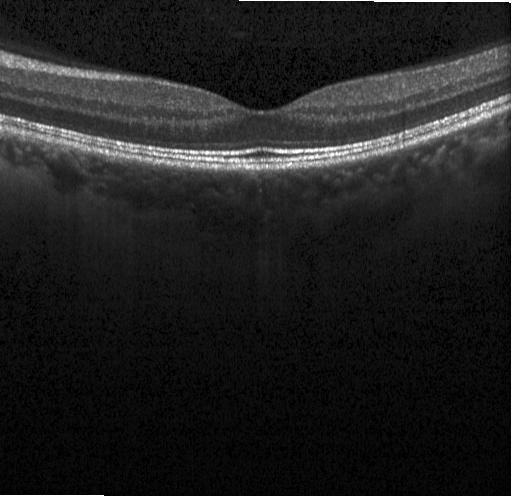 OCT line scan. Assessment: no choroidal neovascularization, no diabetic macular edema, and no drusen.